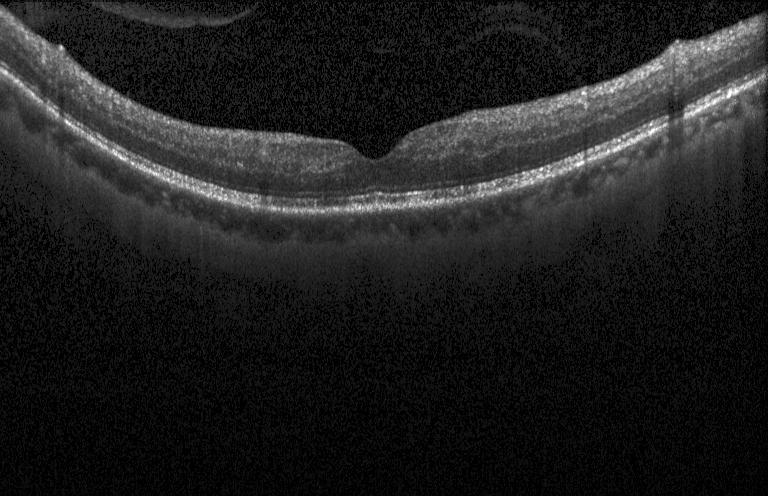 Diagnosis: neither choroidal neovascularization, diabetic macular edema, nor drusen.